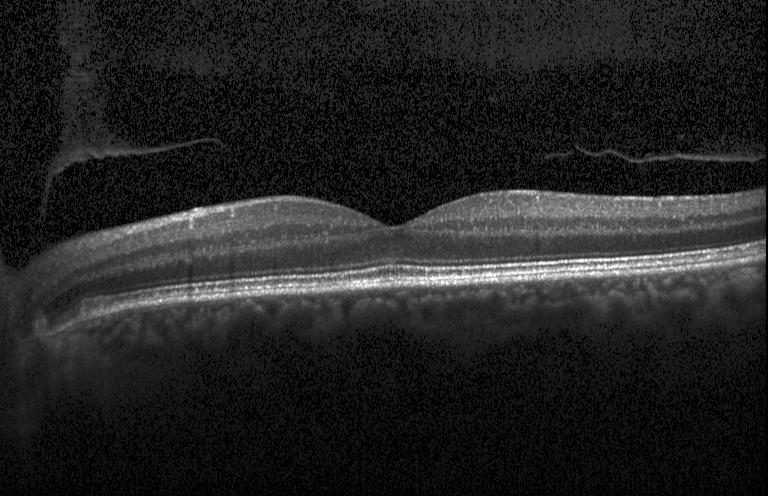

Acquired on a Heidelberg Spectralis; OCT line scan; macular scan
The scan shows neither CNV, DME, nor drusen.